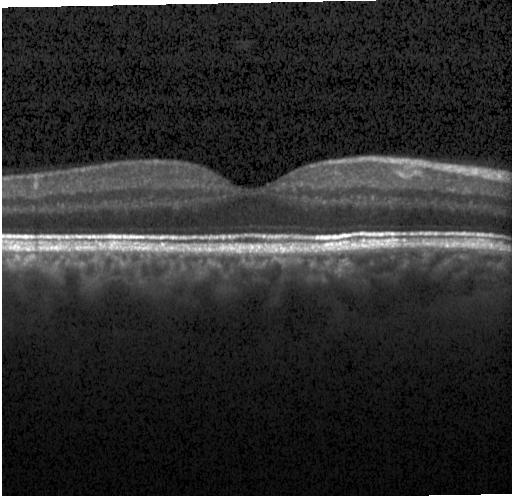
Heidelberg Spectralis; OCT B-scan; horizontal scan through the fovea; SD-OCT — This B-scan demonstrates neither choroidal neovascularization, diabetic macular edema, nor drusen.